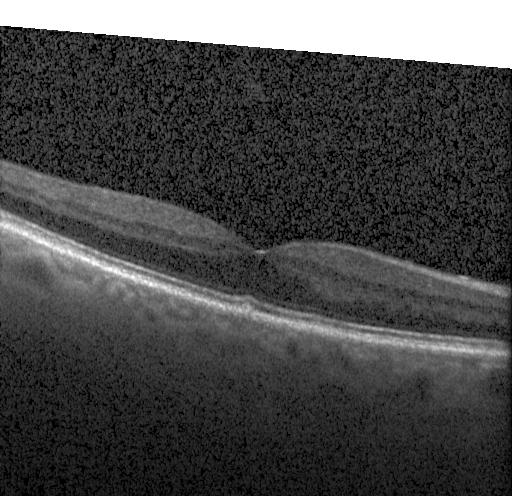

SD-OCT; retinal OCT B-scan; acquired on a Heidelberg Spectralis. Impression: no CNV, DME, or drusen.